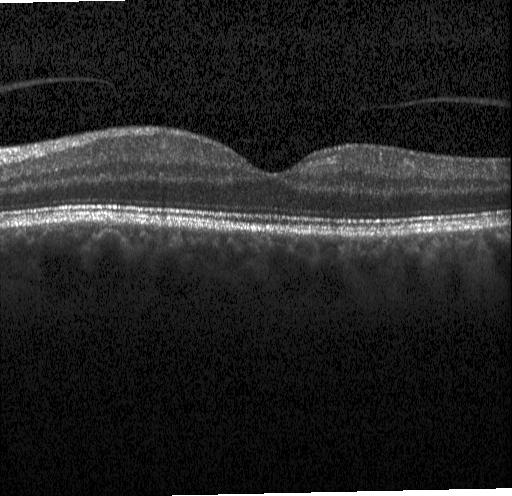

This B-scan demonstrates neither CNV, DME, nor drusen.